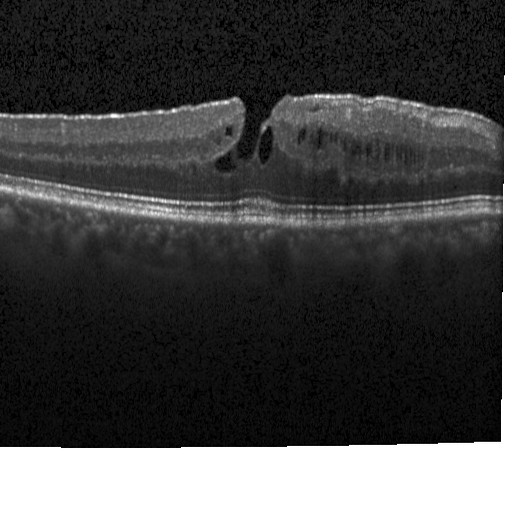 Fovea-centered; Heidelberg Spectralis OCT system; retinal OCT B-scan. This B-scan demonstrates DME.